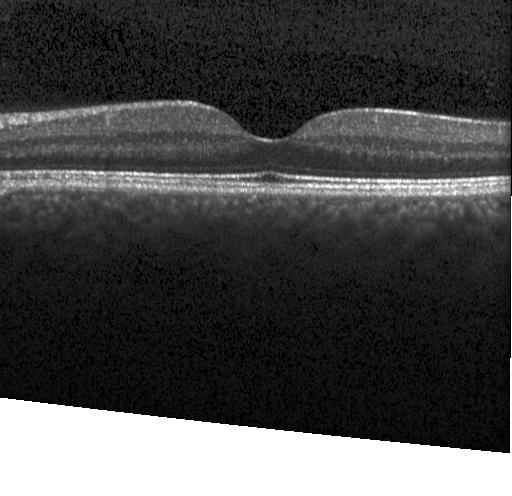
Retinal OCT B-scan.
Macular OCT: no choroidal neovascularization, no diabetic macular edema, and no drusen.